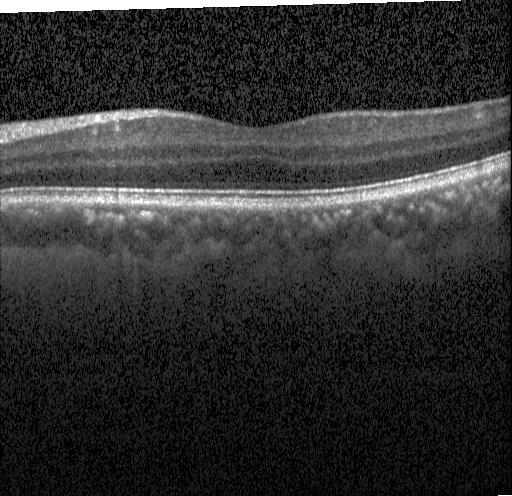

Impression: neither choroidal neovascularization, diabetic macular edema, nor drusen.